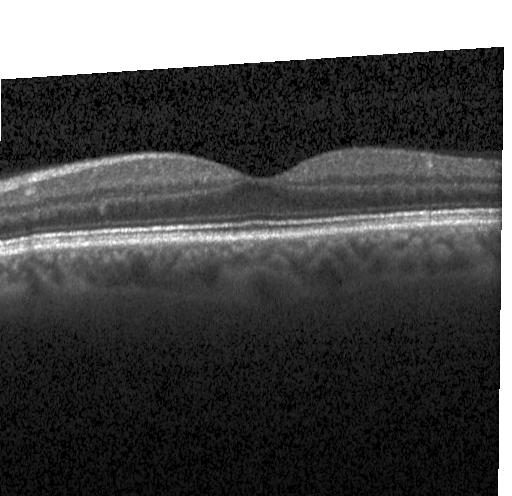 OCT B-scan showing no CNV, DME, or drusen.